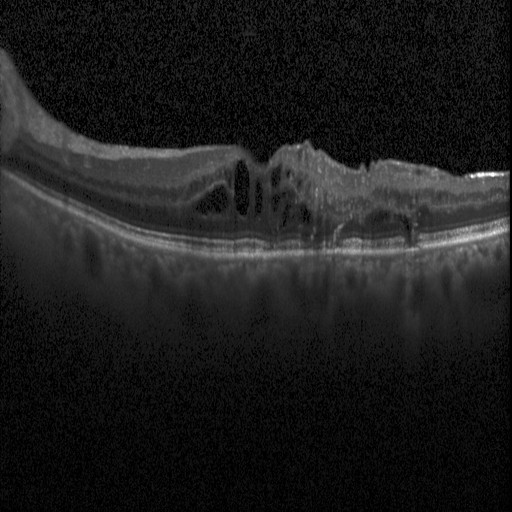

SD-OCT; OCT B-scan; Heidelberg Spectralis OCT system; centered on the fovea. Diagnosis: diabetic macular edema (DME).